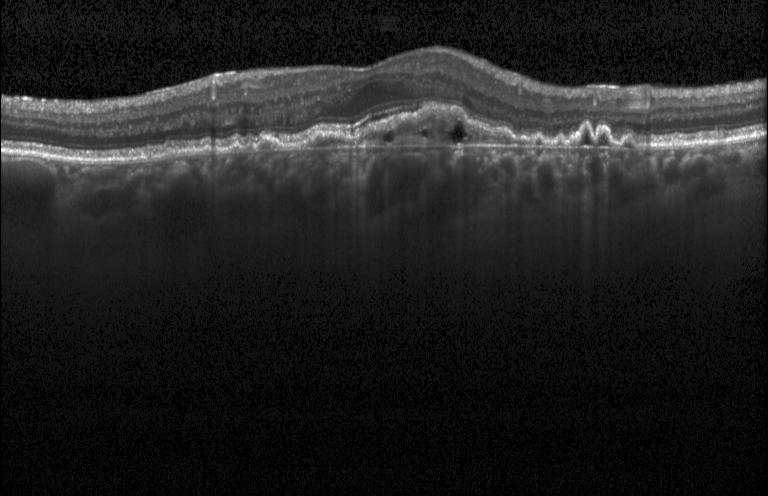 Retinal OCT B-scan.
Finding: a choroidal neovascular membrane.